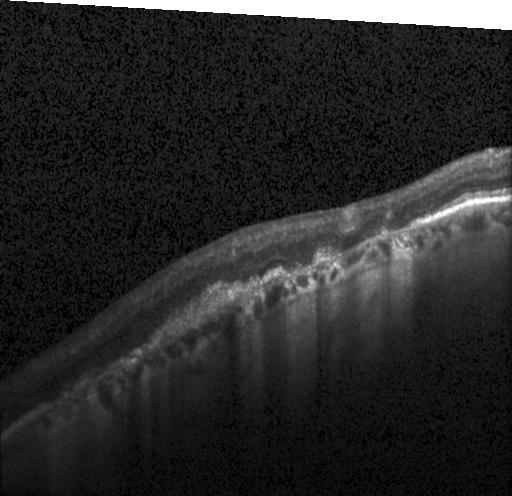
Dx: a choroidal neovascular membrane.